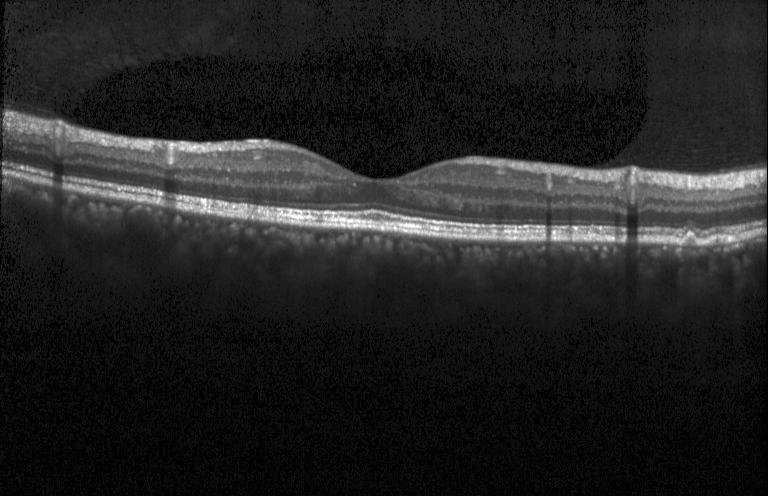

SD-OCT; retinal OCT B-scan; fovea-centered
OCT finding: drusen.